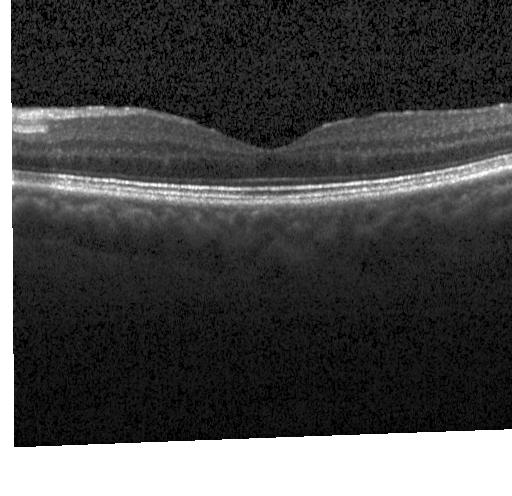

Optical coherence tomography B-scan — Assessment: no CNV, DME, or drusen.